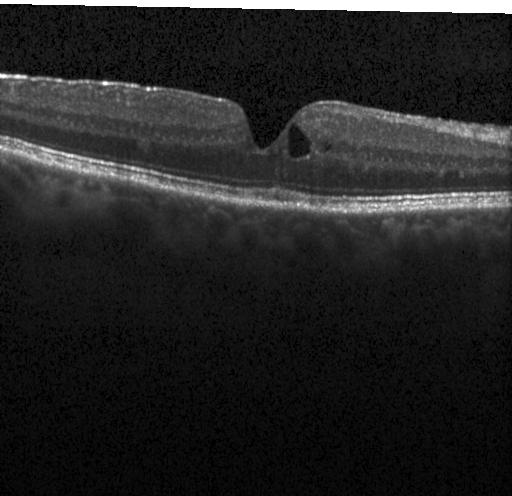

Heidelberg Spectralis OCT system, optical coherence tomography scan, spectral-domain OCT.
Diabetic macular edema (DME).